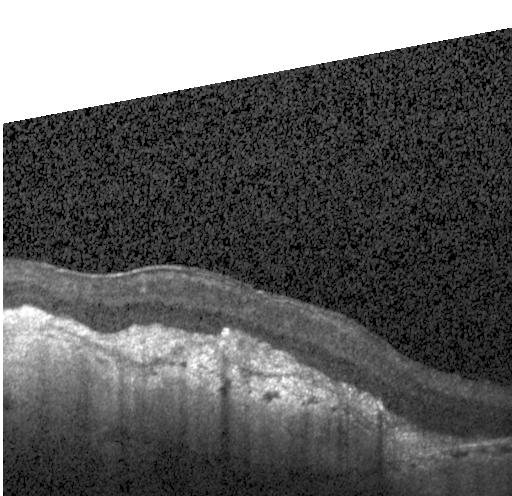

Optical coherence tomography scan. Fovea-centered. SD-OCT.
Finding: a choroidal neovascular membrane.